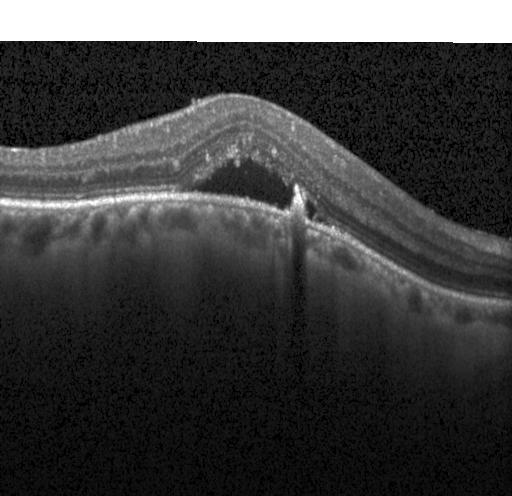

Choroidal neovascularization (CNV).